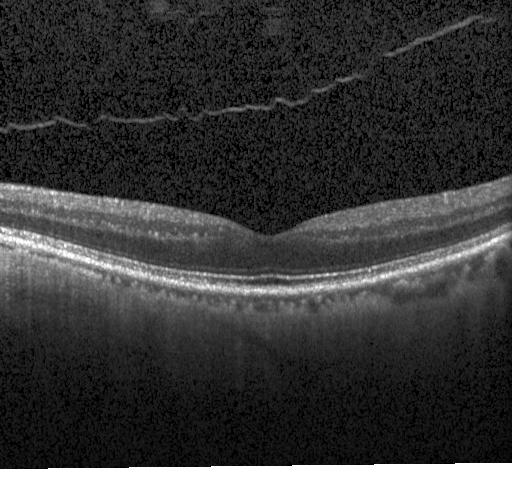
OCT scan showing no choroidal neovascularization, diabetic macular edema, or drusen.